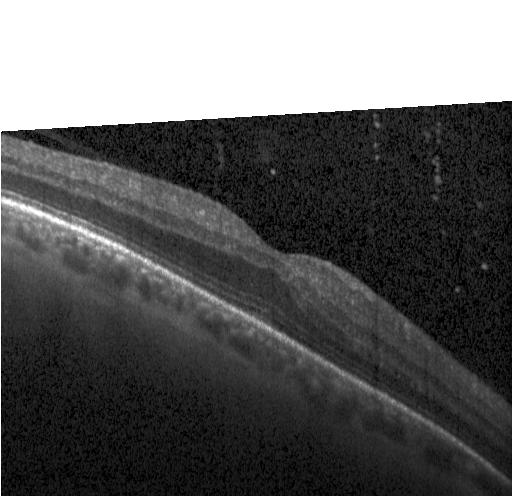

Spectral-domain OCT B-scan: no evidence of choroidal neovascularization, diabetic macular edema, or drusen.